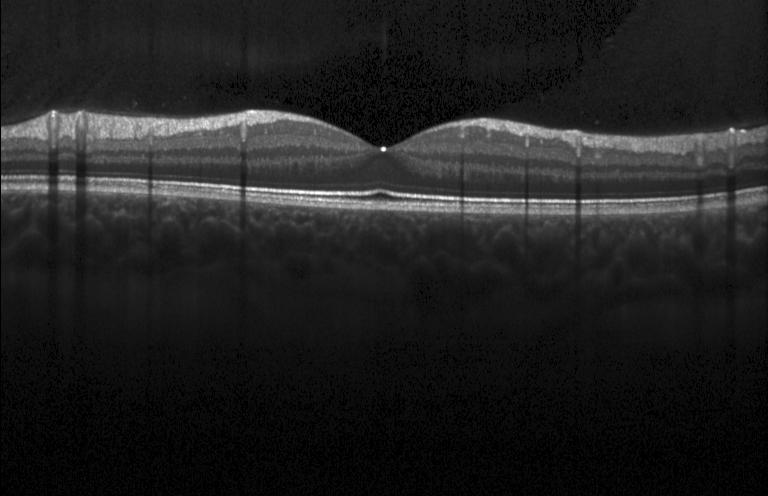

OCT scan showing no choroidal neovascularization, no diabetic macular edema, and no drusen.